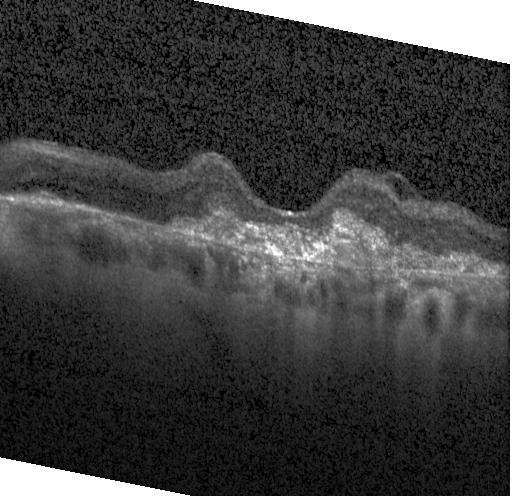
Fovea-centered; OCT line scan
Dx: a choroidal neovascular membrane.